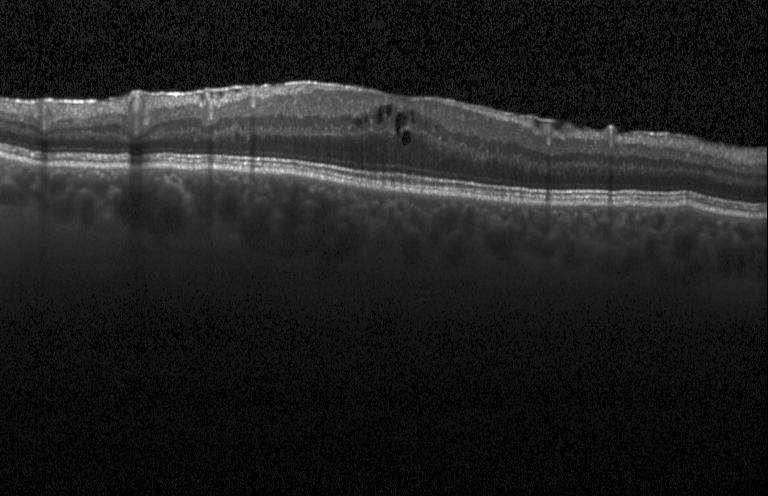 Diabetic macular edema (DME).